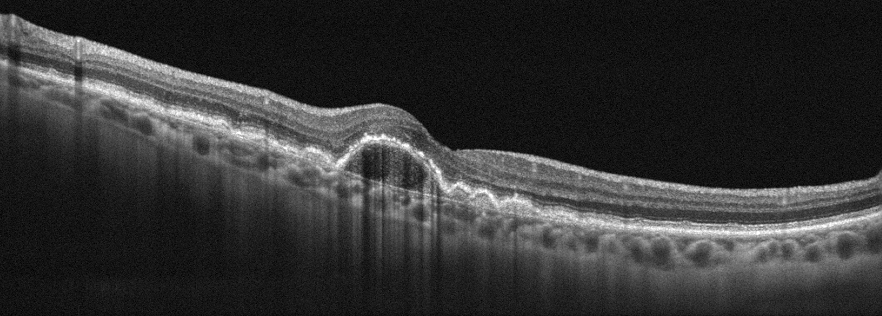

Left eye · retinal OCT B-scan · fovea-centered
Diagnosis: age-related macular degeneration (AMD).